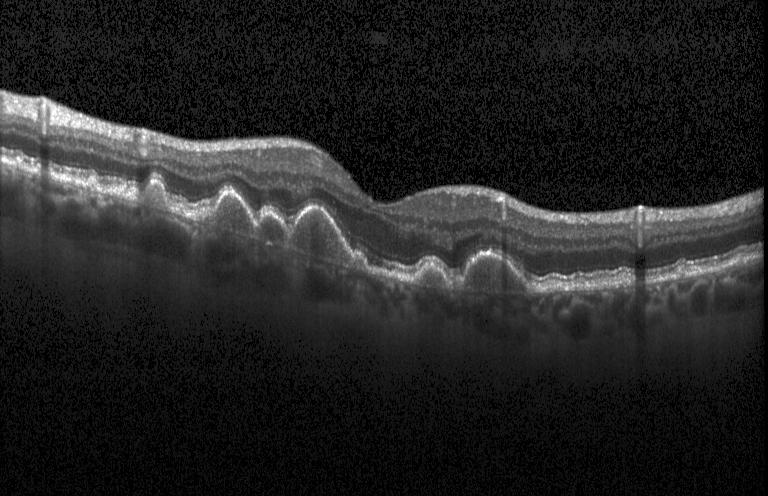

OCT B-scan. Spectral-domain OCT. Macular scan. Acquired on a Heidelberg Spectralis.
OCT finding: sub-RPE drusenoid deposits.